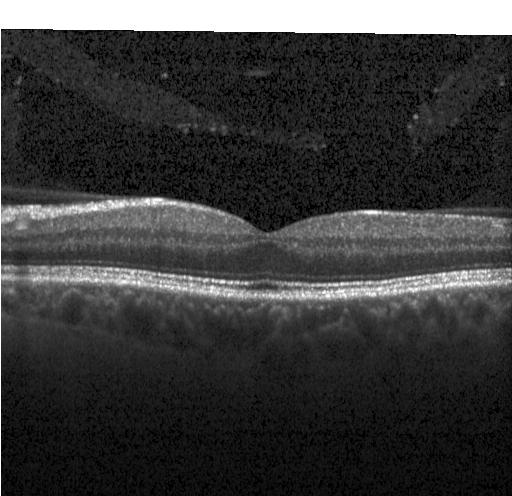
OCT B-scan · centered on the fovea · acquired on a Heidelberg Spectralis · SD-OCT.
Diagnosis: no choroidal neovascularization, no diabetic macular edema, and no drusen.